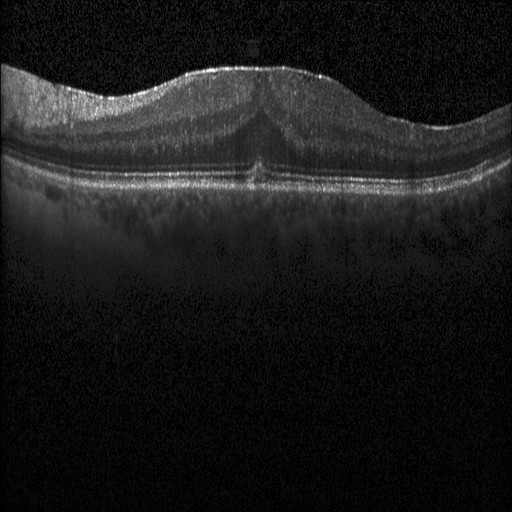

Impression: diabetic macular edema.